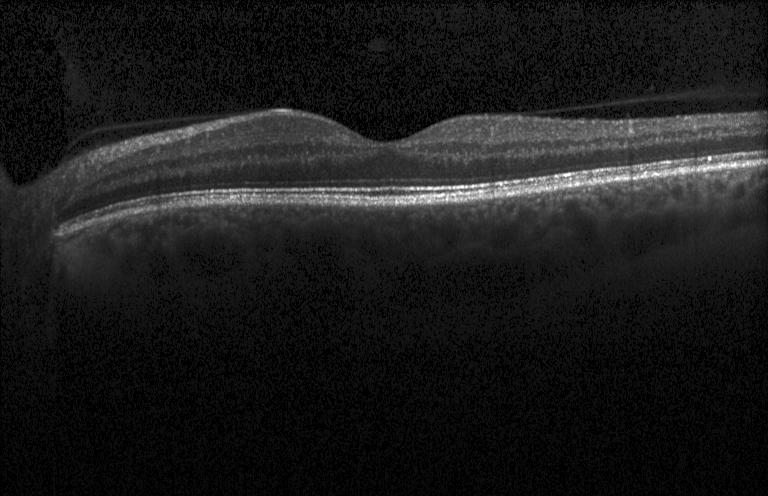
Macular OCT demonstrating no CNV, no DME, and no drusen.